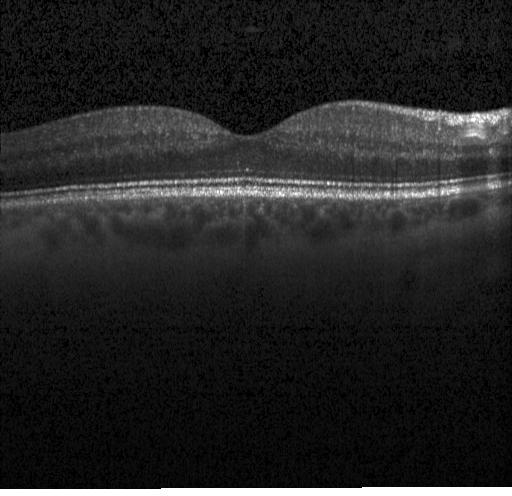

The scan shows neither CNV, DME, nor drusen.